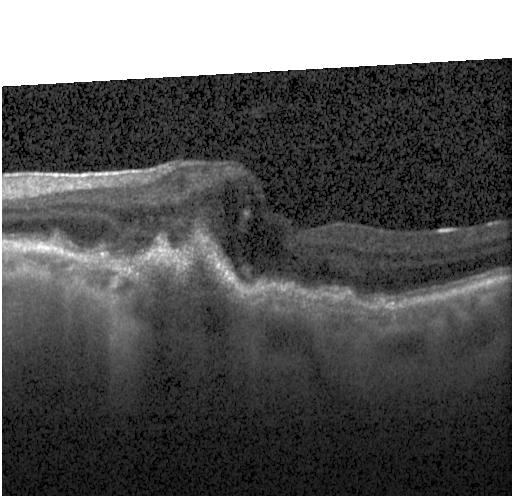

SD-OCT. Centered on the fovea. Optical coherence tomography scan — Finding: choroidal neovascularization (CNV).